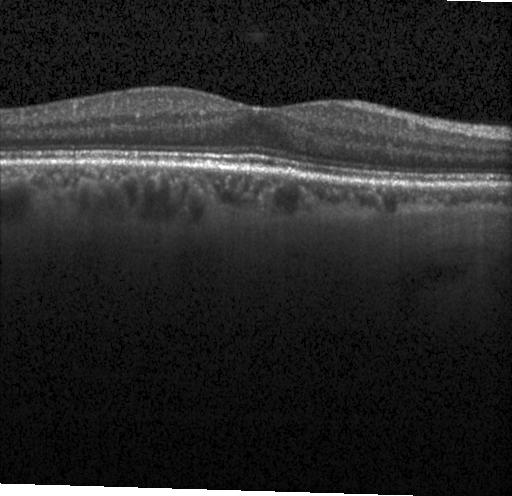
Retinal OCT B-scan.
This B-scan demonstrates no choroidal neovascularization, no diabetic macular edema, and no drusen.